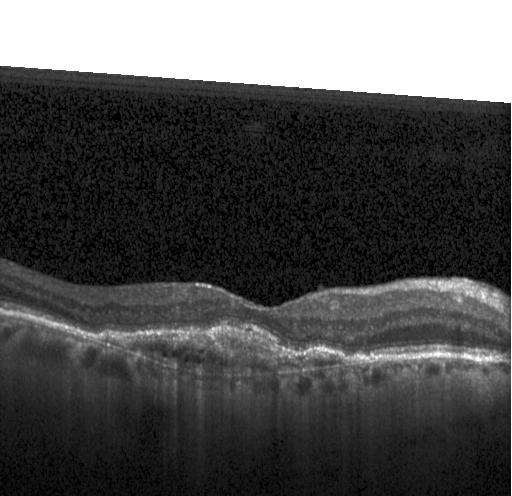 Retinal OCT cross-section.
A choroidal neovascular membrane.